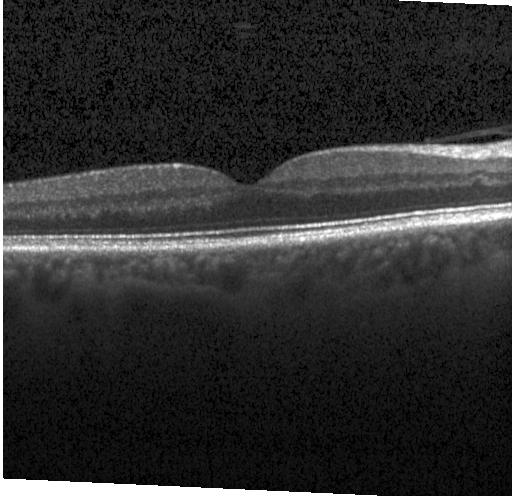

Instrument: Heidelberg Spectralis; through the macula; spectral-domain OCT; optical coherence tomography scan — Assessment: no evidence of choroidal neovascularization, diabetic macular edema, or drusen.